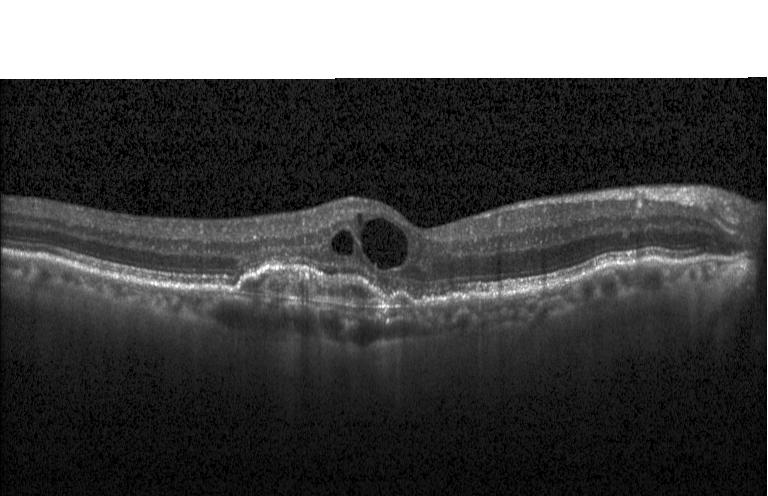

Impression: choroidal neovascularization (CNV).